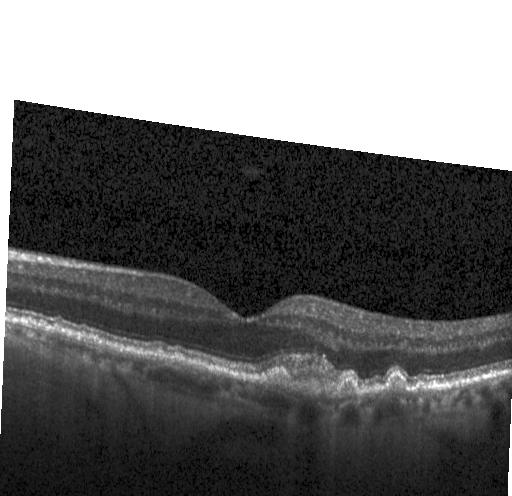 Retinal OCT cross-section
Assessment: a choroidal neovascular membrane.